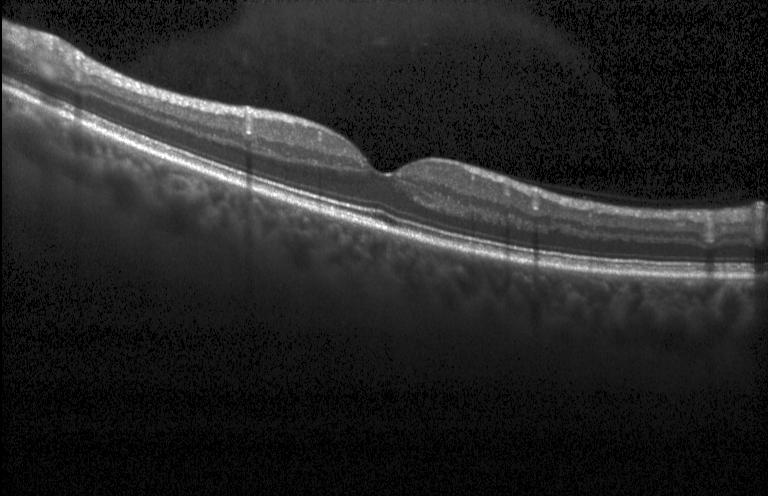 Finding: no choroidal neovascularization, no diabetic macular edema, and no drusen.